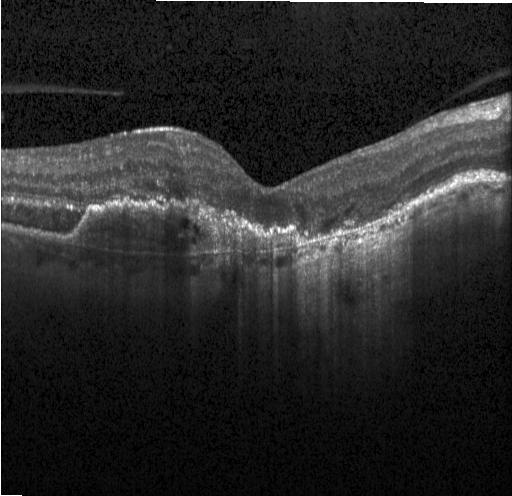
Macular scan; SD-OCT; OCT line scan. Finding: choroidal neovascularization.